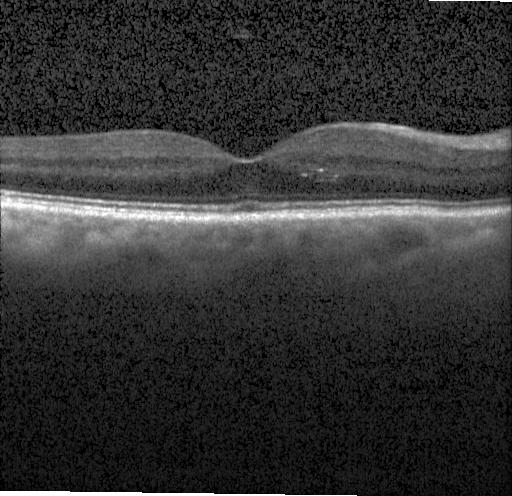 OCT B-scan showing no evidence of choroidal neovascularization, diabetic macular edema, or drusen.